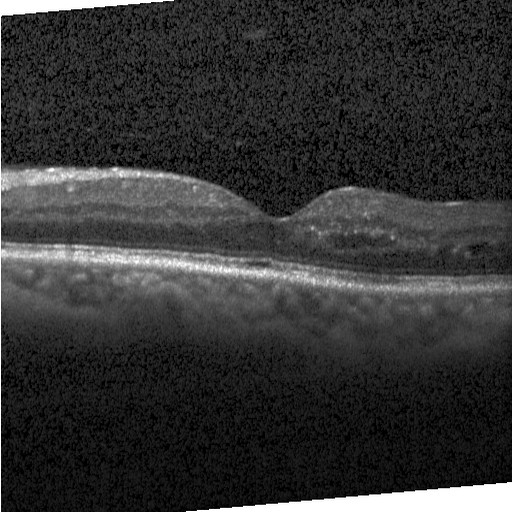

OCT B-scan.
Impression: diabetic macular edema.